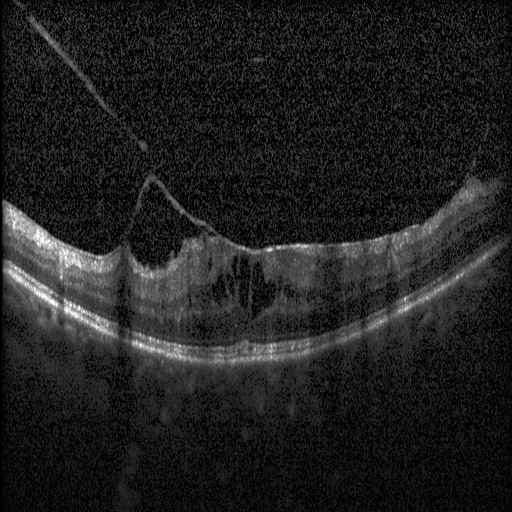

Impression: diabetic macular edema.